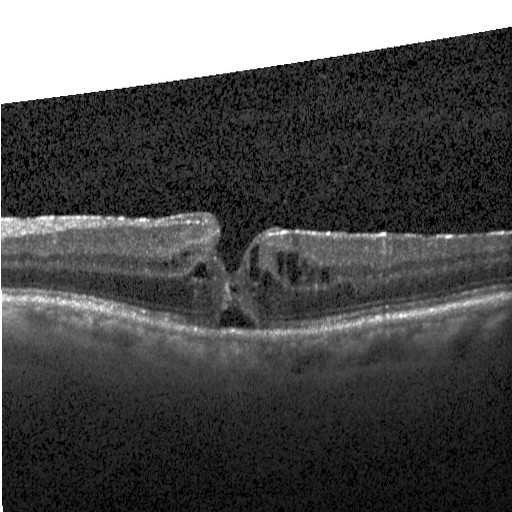

Acquired on a Heidelberg Spectralis. Retinal OCT B-scan
OCT finding: diabetic macular edema.